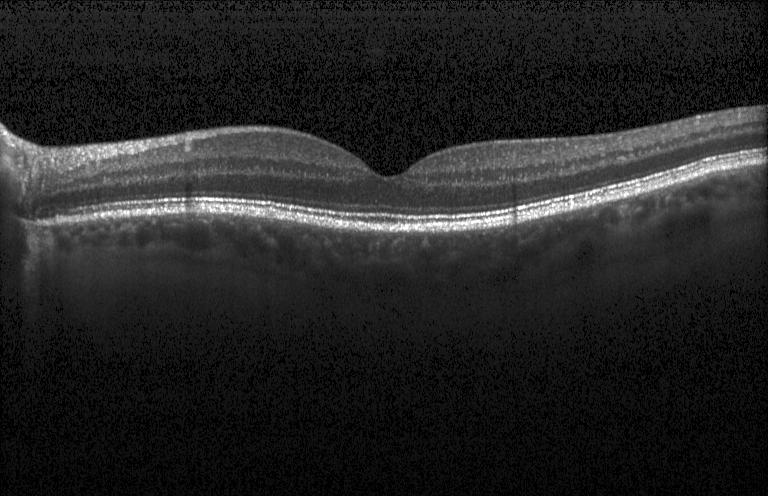 Optical coherence tomography scan · spectral-domain OCT. Macular OCT: no CNV, DME, or drusen.